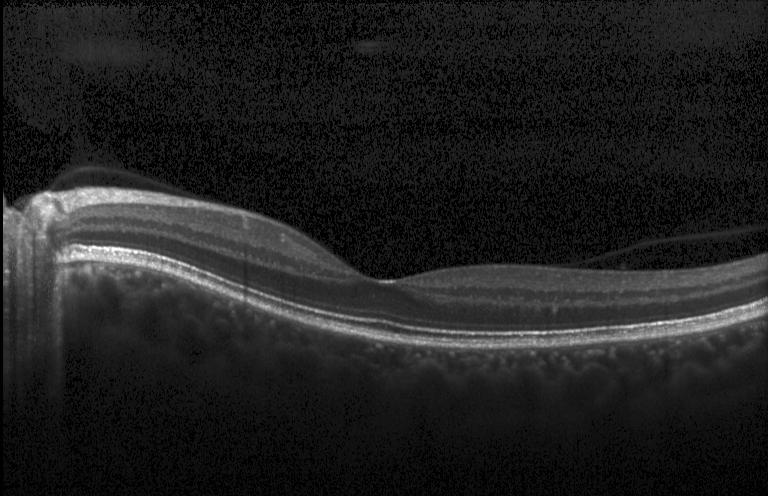
Neither CNV, DME, nor drusen.